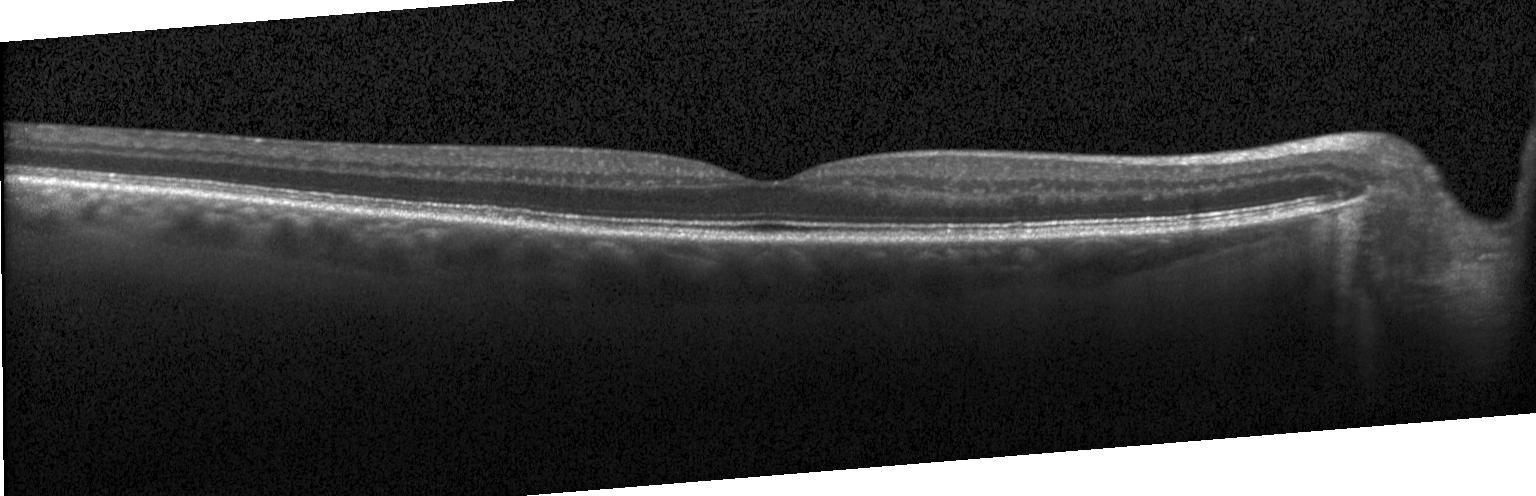

Retinal OCT B-scan
OCT finding: neither choroidal neovascularization, diabetic macular edema, nor drusen.